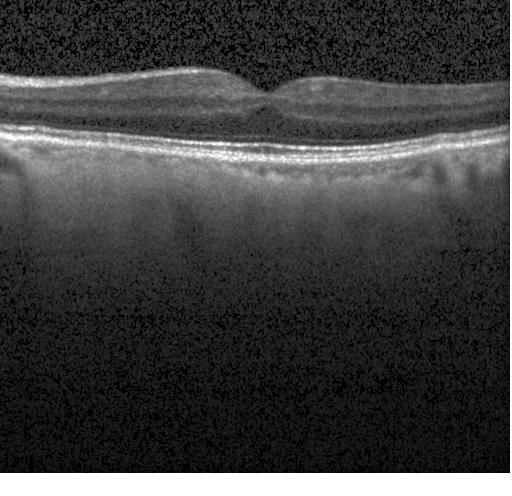 Spectral-domain optical coherence tomography; optical coherence tomography B-scan; macular scan.
OCT finding: no choroidal neovascularization, no diabetic macular edema, and no drusen.